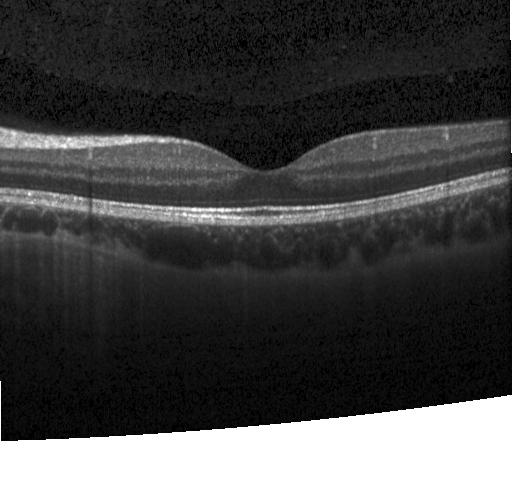
OCT B-scan — Diagnosis: no evidence of choroidal neovascularization, diabetic macular edema, or drusen.